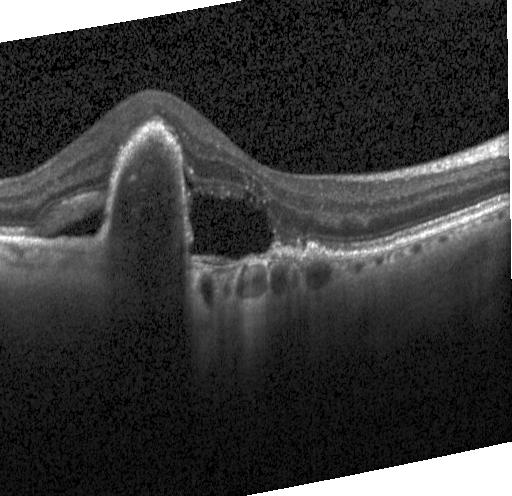
Acquired on a Heidelberg Spectralis. Retinal OCT B-scan — Macular OCT: a choroidal neovascular membrane.